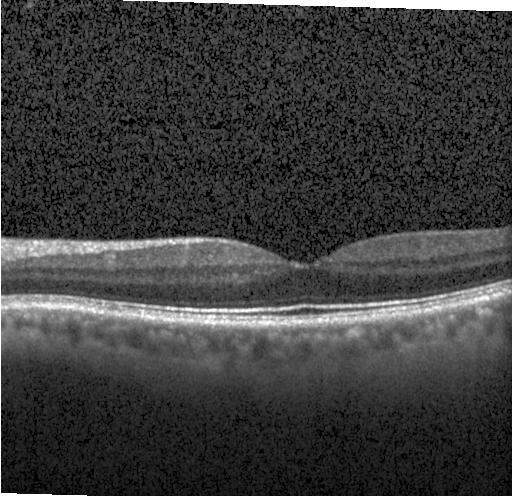 Macular OCT demonstrating no choroidal neovascularization, no diabetic macular edema, and no drusen.